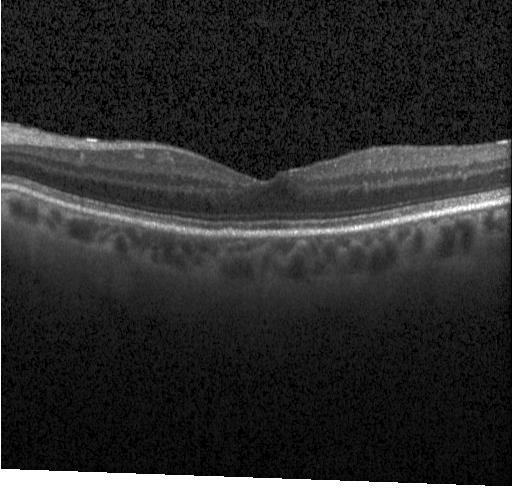 OCT B-scan showing no evidence of choroidal neovascularization, diabetic macular edema, or drusen.